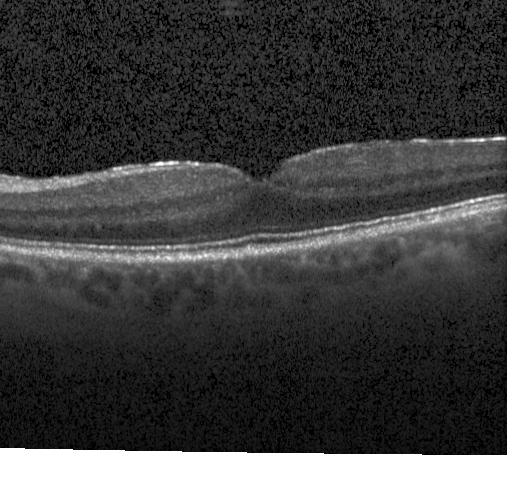

Optical coherence tomography scan — Impression: no choroidal neovascularization, no diabetic macular edema, and no drusen.